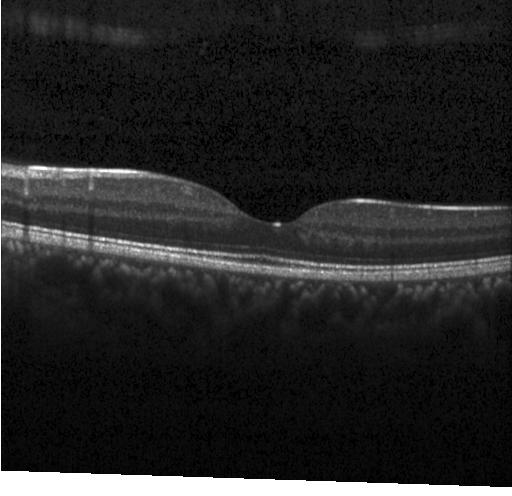
Heidelberg Spectralis; fovea-centered; retinal OCT B-scan
Diagnosis: no CNV, no DME, and no drusen.